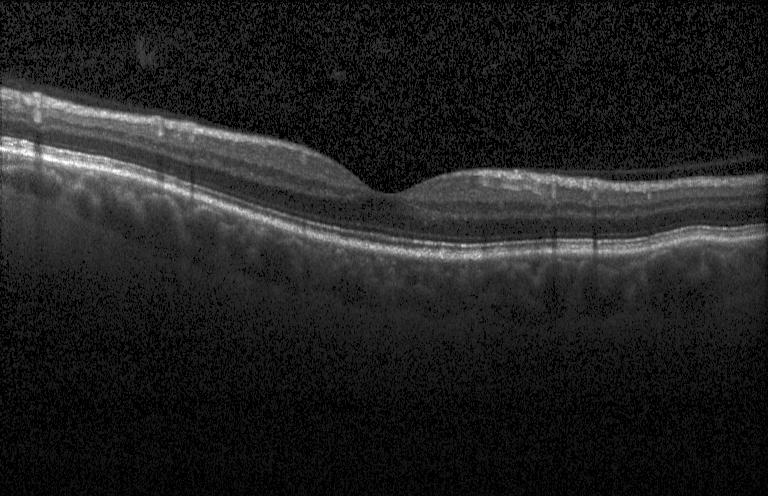

Finding: neither CNV, DME, nor drusen.